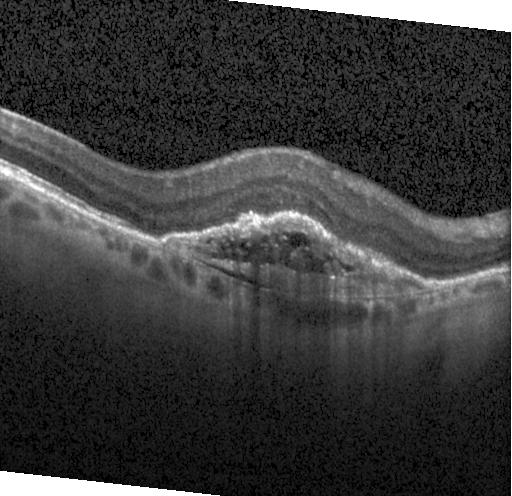

Heidelberg Spectralis · SD-OCT · OCT B-scan — OCT finding: a choroidal neovascular membrane.